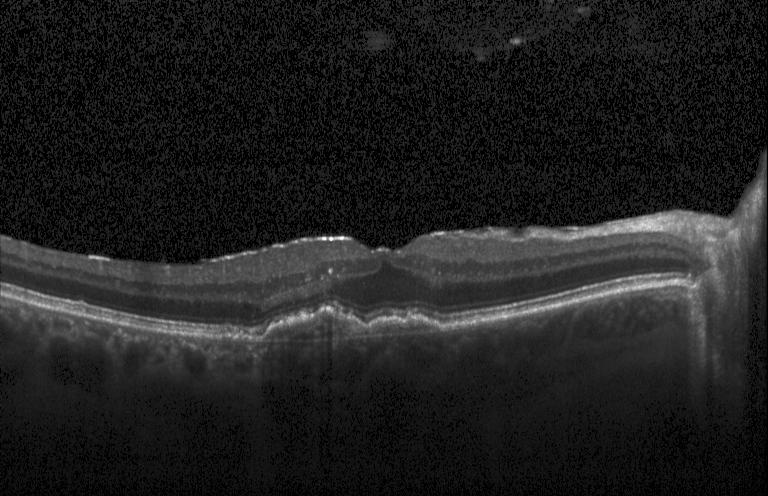
Macular scan. OCT B-scan. Heidelberg Spectralis OCT system
Dx: CNV.